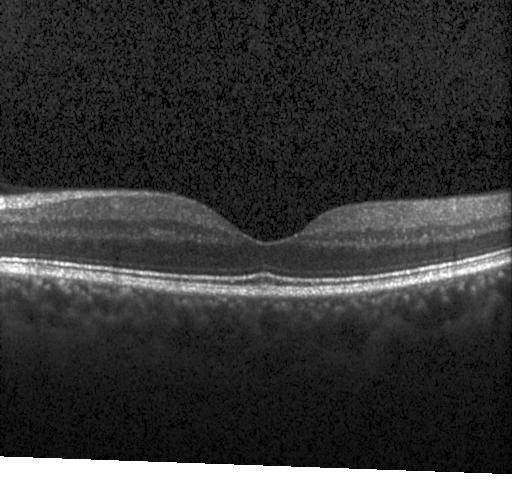 Heidelberg Spectralis. SD-OCT. OCT line scan
Assessment: no choroidal neovascularization, no diabetic macular edema, and no drusen.